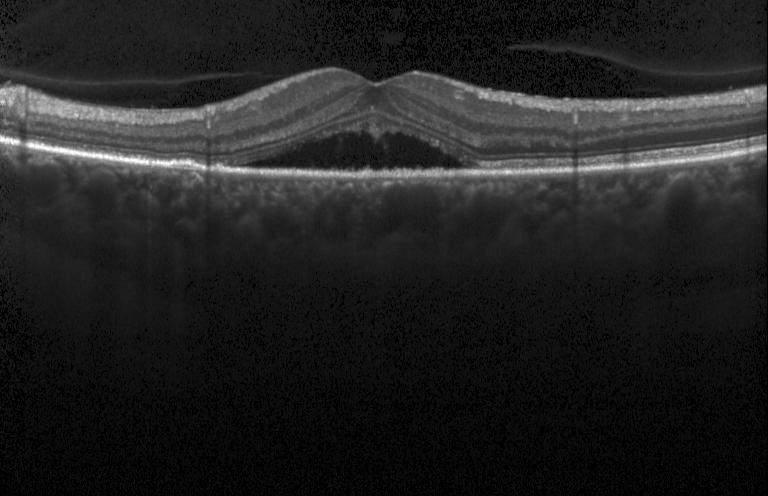
Optical coherence tomography scan. Through the macula. Spectral-domain OCT. Finding: a choroidal neovascular membrane.